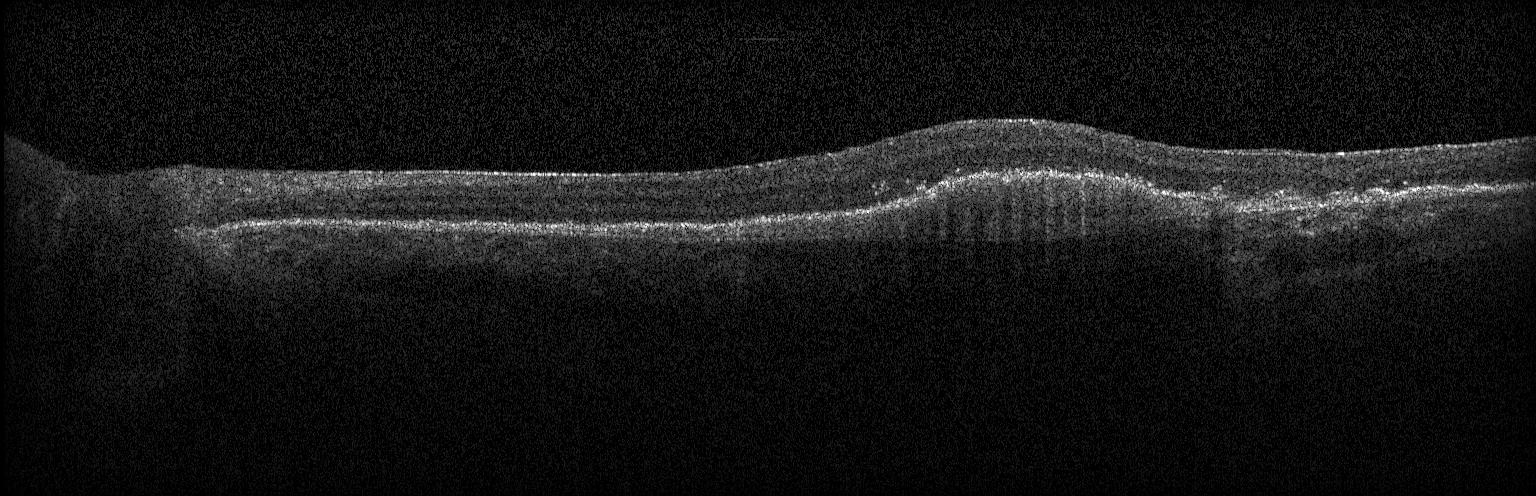

Spectral-domain OCT · fovea-centered · Heidelberg Spectralis OCT system · retinal OCT cross-section. A choroidal neovascular membrane.